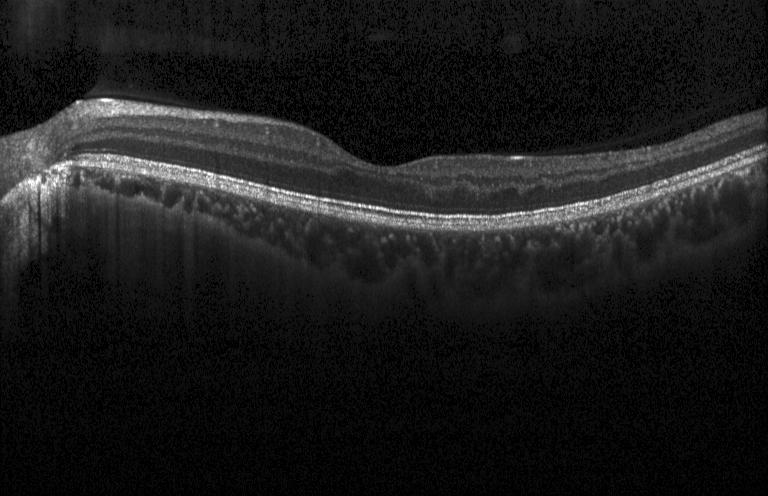

Spectral-domain OCT · OCT line scan · Heidelberg Spectralis OCT system.
Diagnosis: no choroidal neovascularization, no diabetic macular edema, and no drusen.